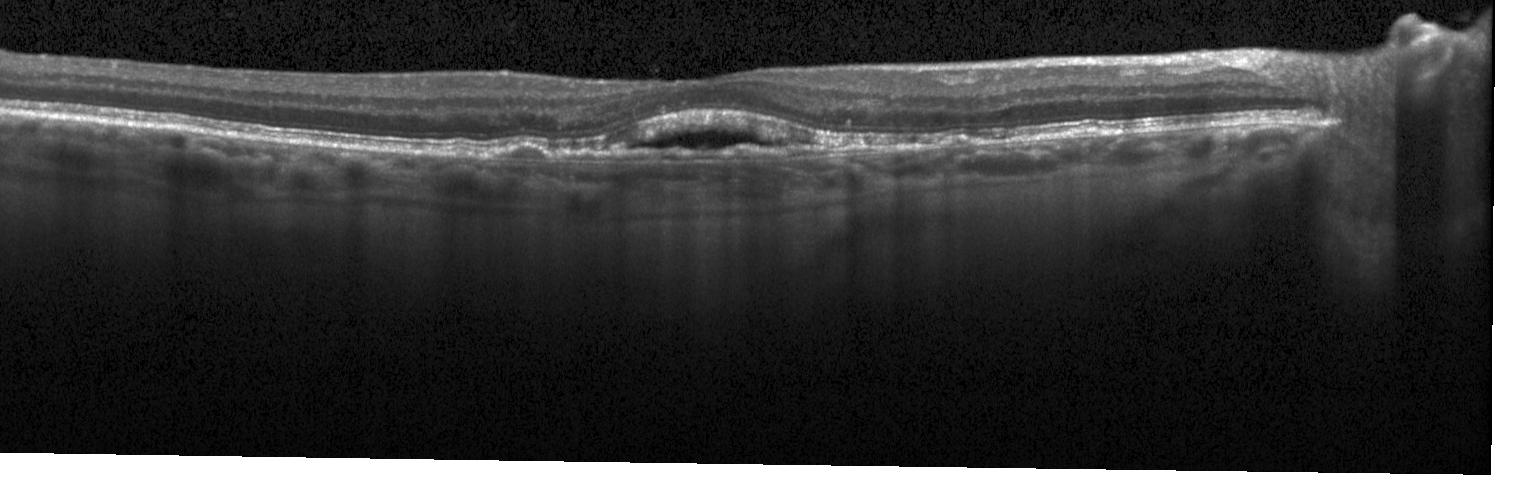
This B-scan demonstrates a choroidal neovascular membrane.